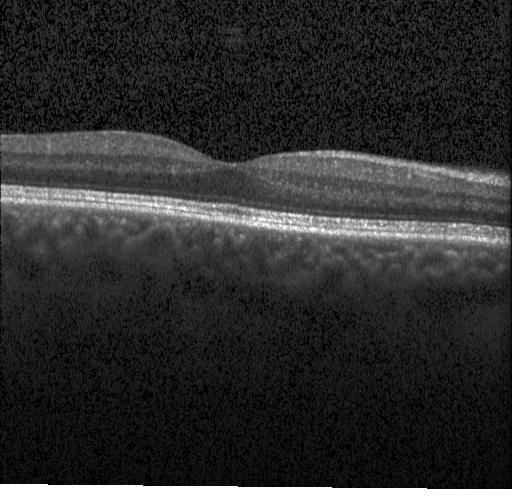 OCT scan showing no choroidal neovascularization, diabetic macular edema, or drusen.